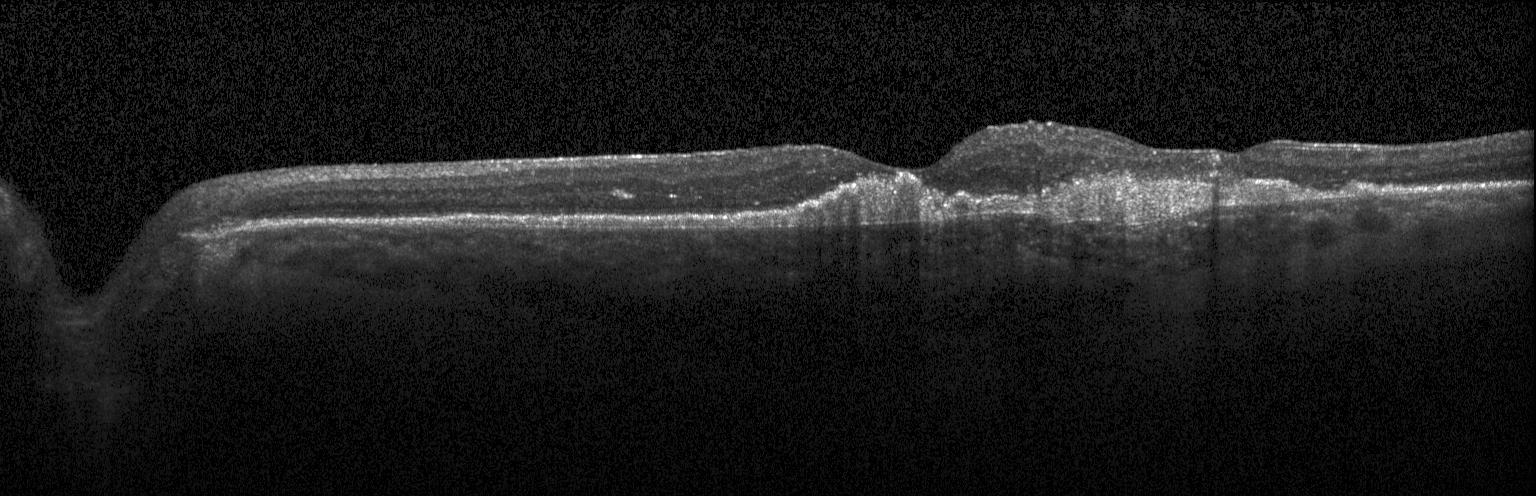
Dx: a choroidal neovascular membrane.